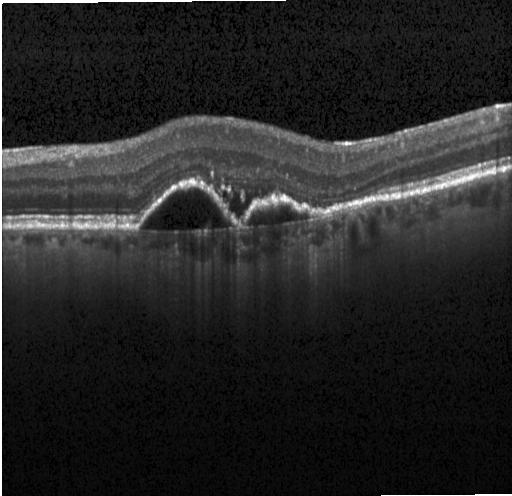 Horizontal scan through the fovea · optical coherence tomography scan · SD-OCT.
Macular OCT: choroidal neovascularization (CNV).